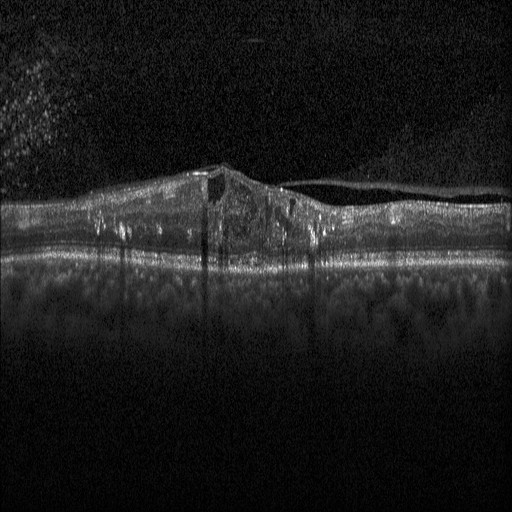 Fovea-centered; instrument: Heidelberg Spectralis; spectral-domain OCT; optical coherence tomography B-scan — Dx: DME.